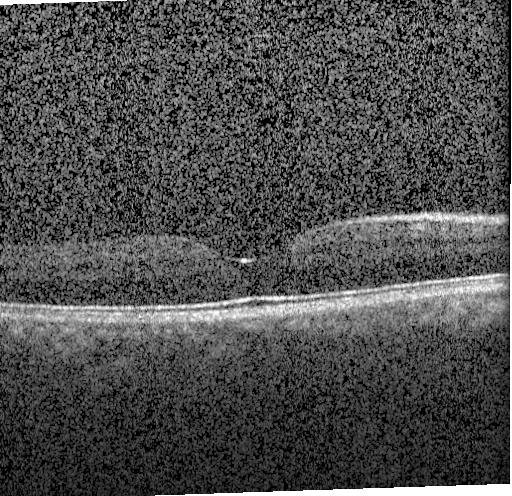 Retinal OCT B-scan. Diagnosis: no CNV, no DME, and no drusen.